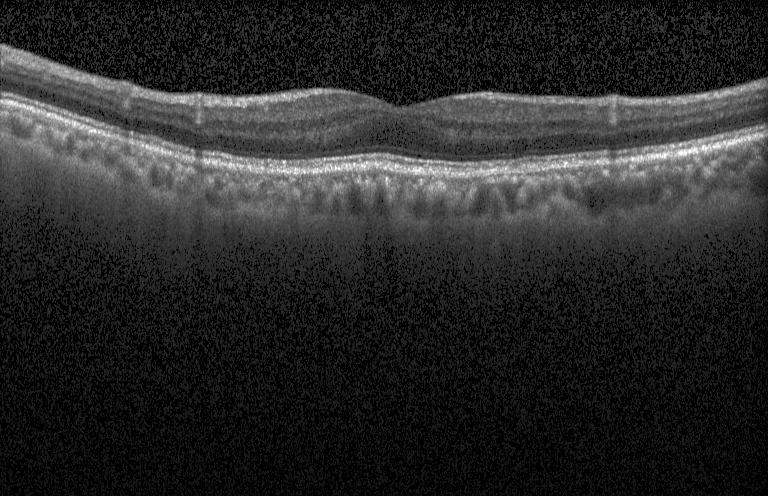

Finding: no evidence of CNV, DME, or drusen.